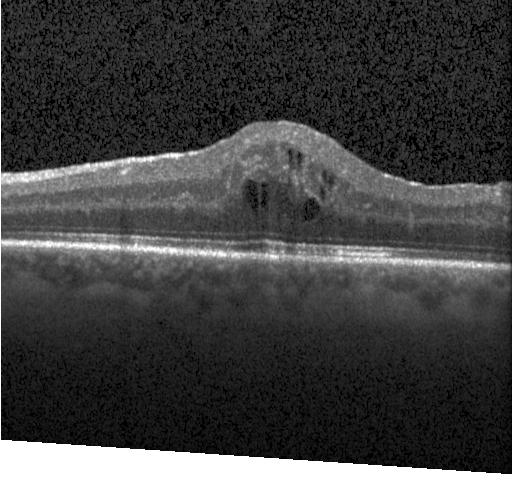 Spectral-domain optical coherence tomography · OCT line scan
Macular OCT: diabetic macular edema (DME).